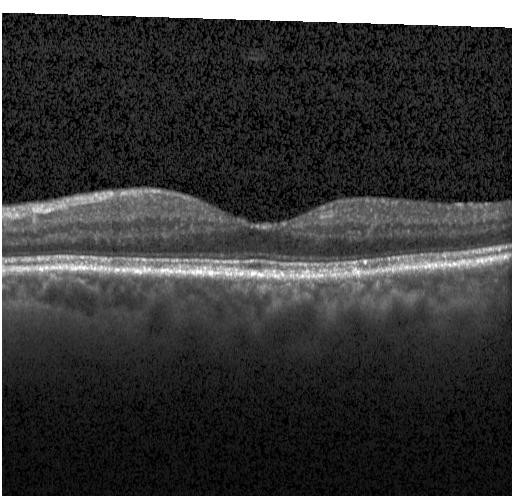 OCT finding: no choroidal neovascularization, no diabetic macular edema, and no drusen.